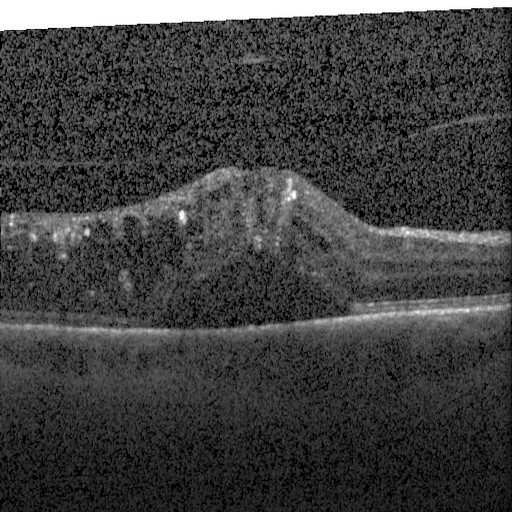

Impression: diabetic macular edema.